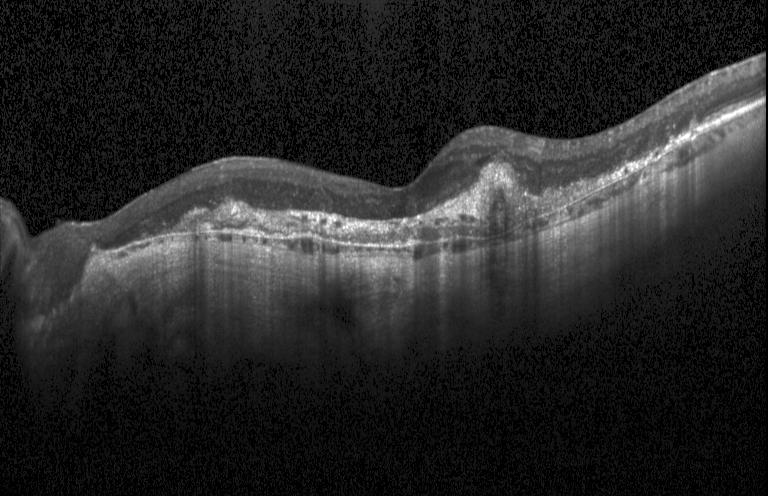
Choroidal neovascularization (CNV).